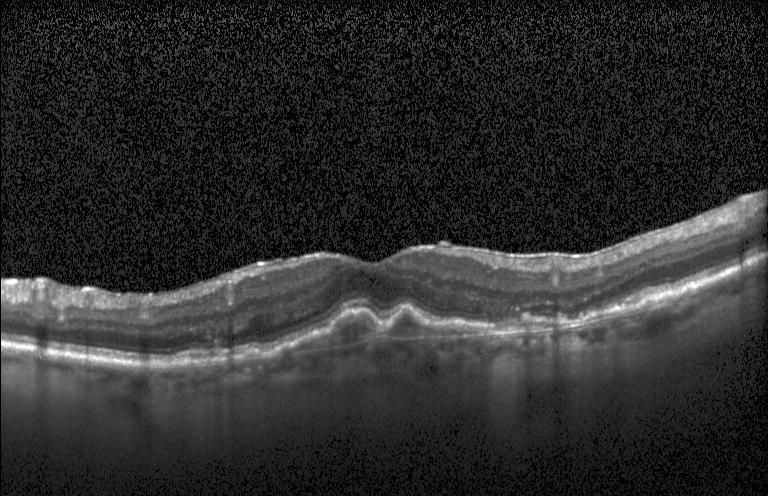
Retinal OCT B-scan
OCT finding: a choroidal neovascular membrane.